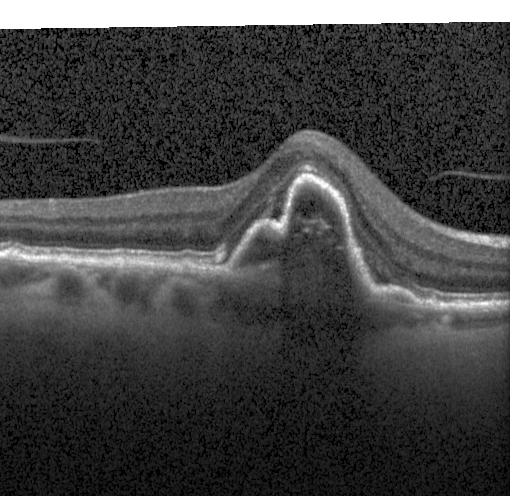 OCT finding: choroidal neovascularization (CNV).